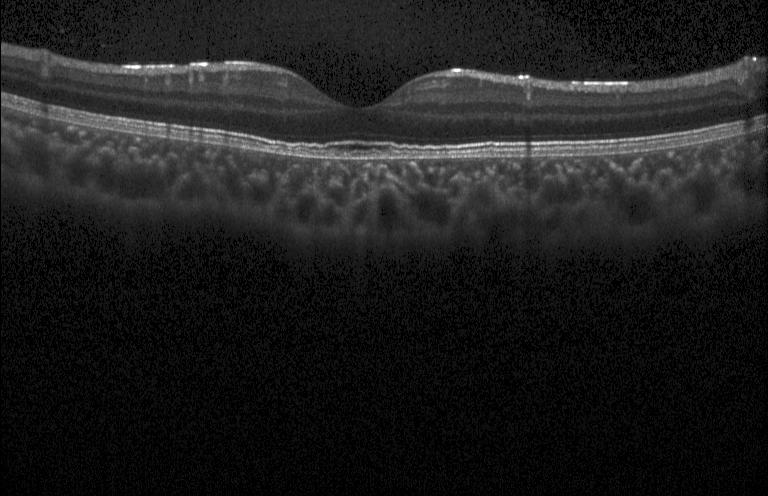

OCT line scan
Impression: no CNV, DME, or drusen.